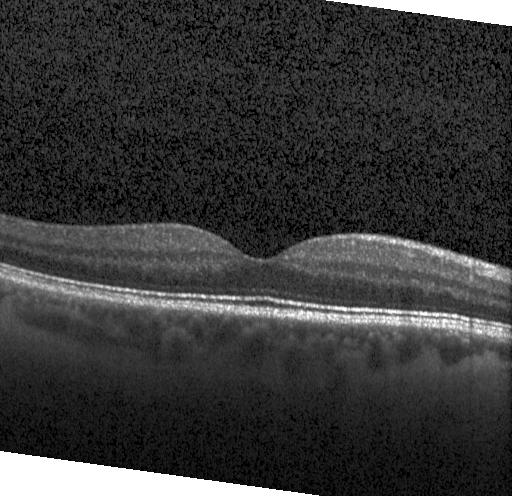
Diagnosis: neither choroidal neovascularization, diabetic macular edema, nor drusen.